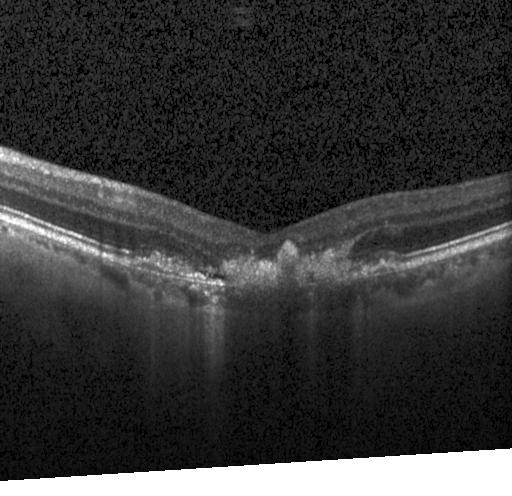 Macular OCT demonstrating choroidal neovascularization.